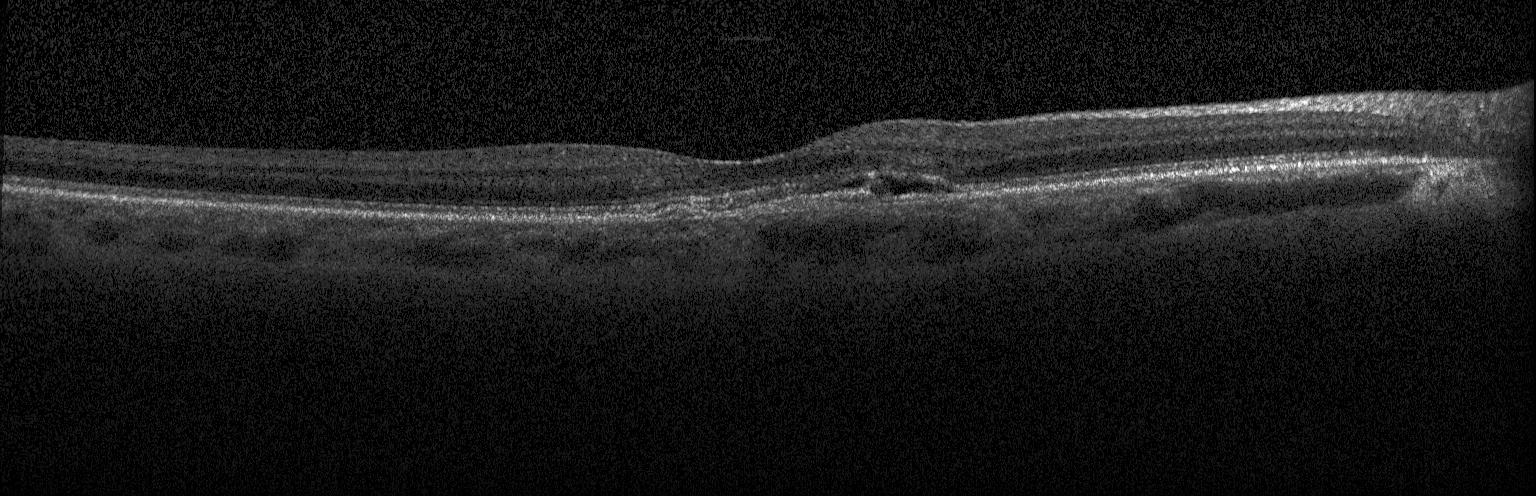 Spectral-domain OCT, optical coherence tomography scan. Macular OCT: a choroidal neovascular membrane.